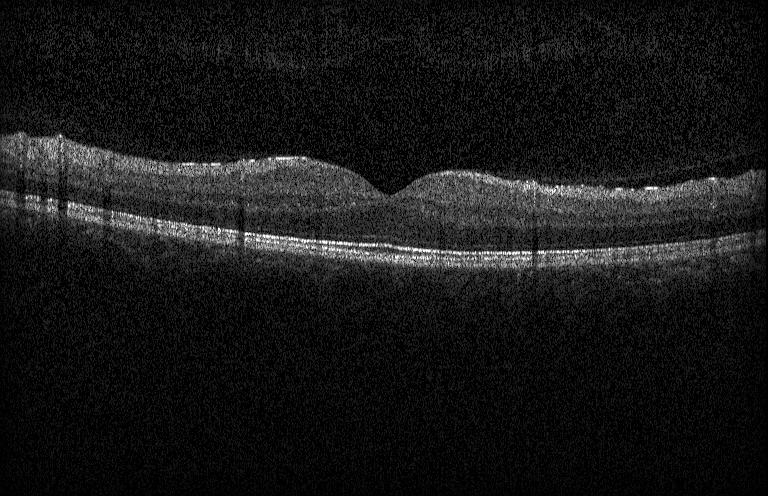

Finding: no choroidal neovascularization, diabetic macular edema, or drusen.